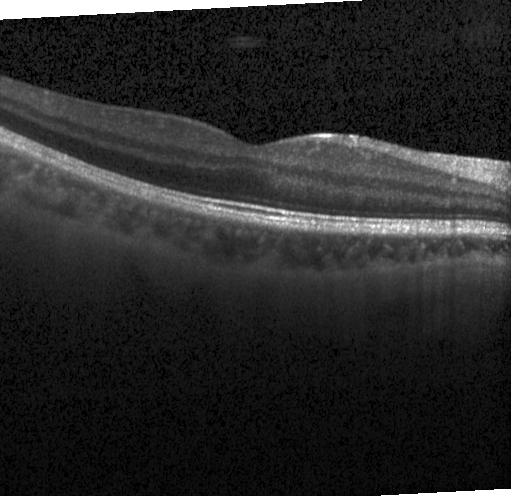

Retinal OCT B-scan, instrument: Heidelberg Spectralis
OCT finding: no evidence of CNV, DME, or drusen.